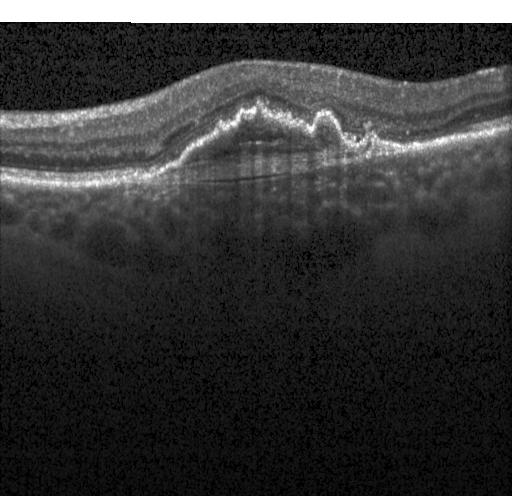
Retinal OCT cross-section, horizontal scan through the fovea — Impression: choroidal neovascularization.